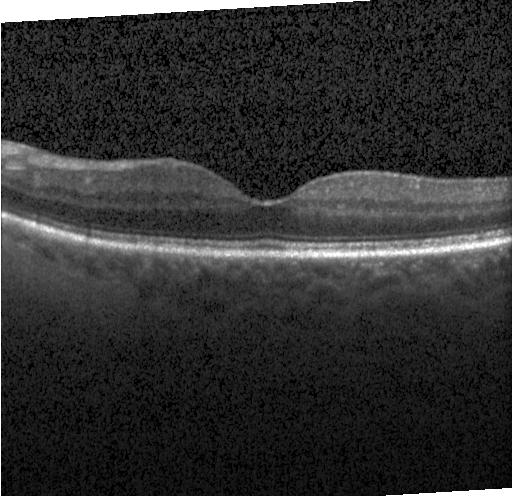

OCT B-scan showing no choroidal neovascularization, diabetic macular edema, or drusen.